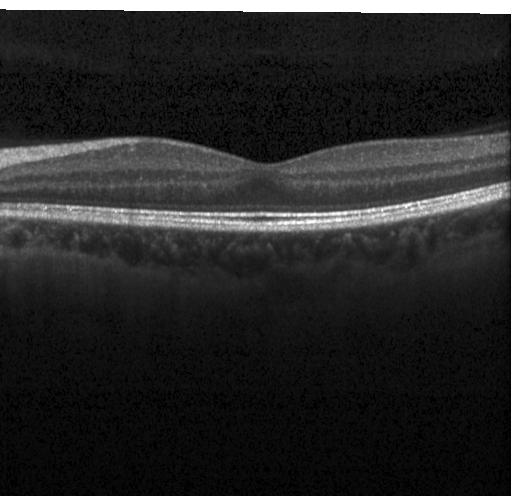 Macular OCT: no CNV, DME, or drusen.